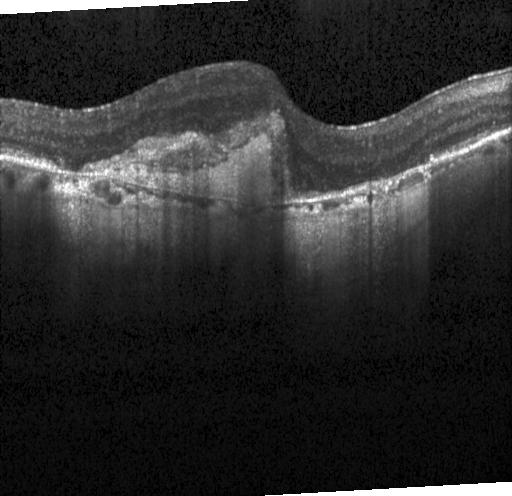

Impression: CNV.